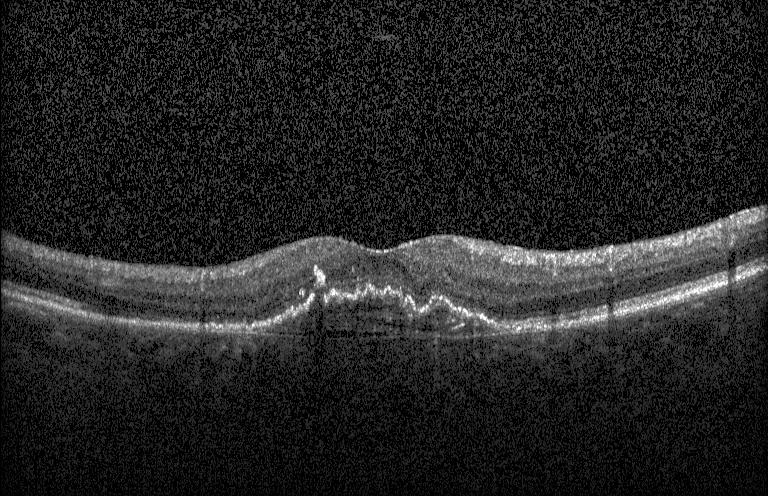

Optical coherence tomography scan.
OCT finding: a choroidal neovascular membrane.